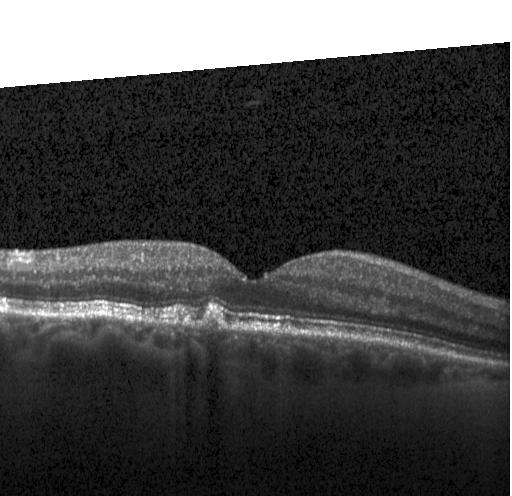 Dx: sub-RPE drusenoid deposits.